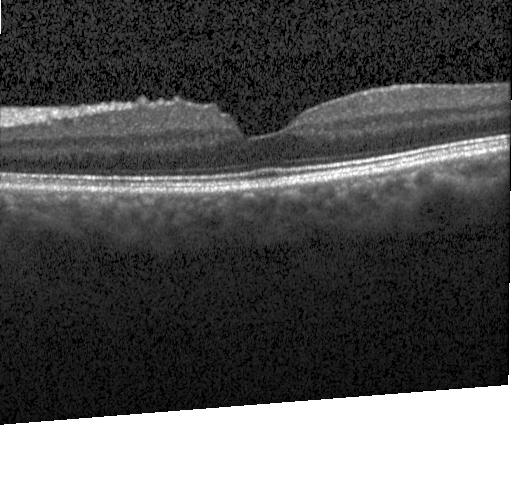
Retinal OCT cross-section.
No CNV, no DME, and no drusen.